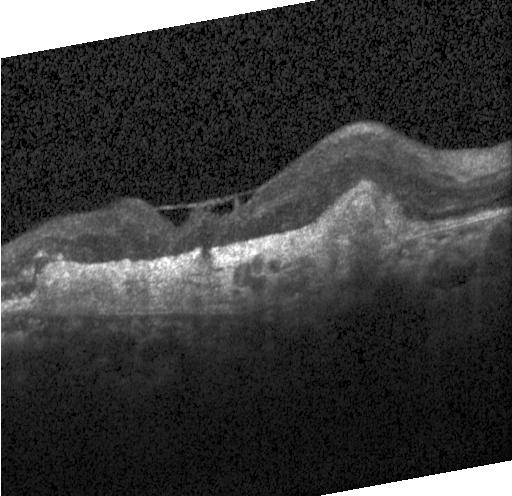 OCT finding: choroidal neovascularization (CNV).